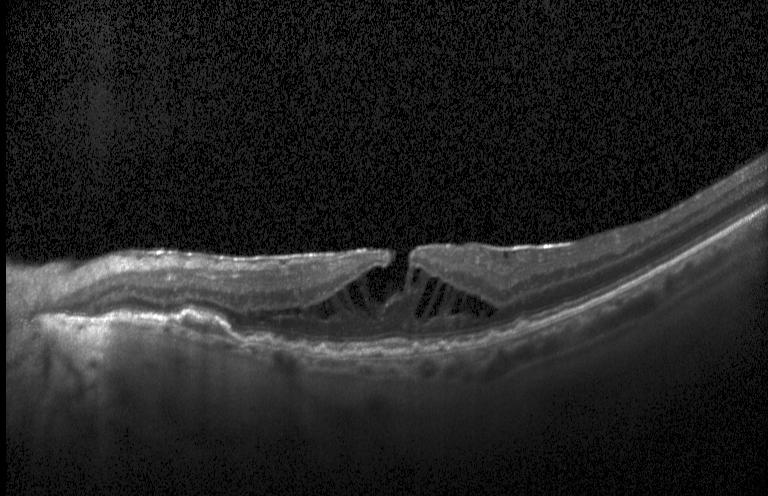
Through the macula. Heidelberg Spectralis. Spectral-domain optical coherence tomography. OCT B-scan
OCT finding: diabetic macular edema (DME).